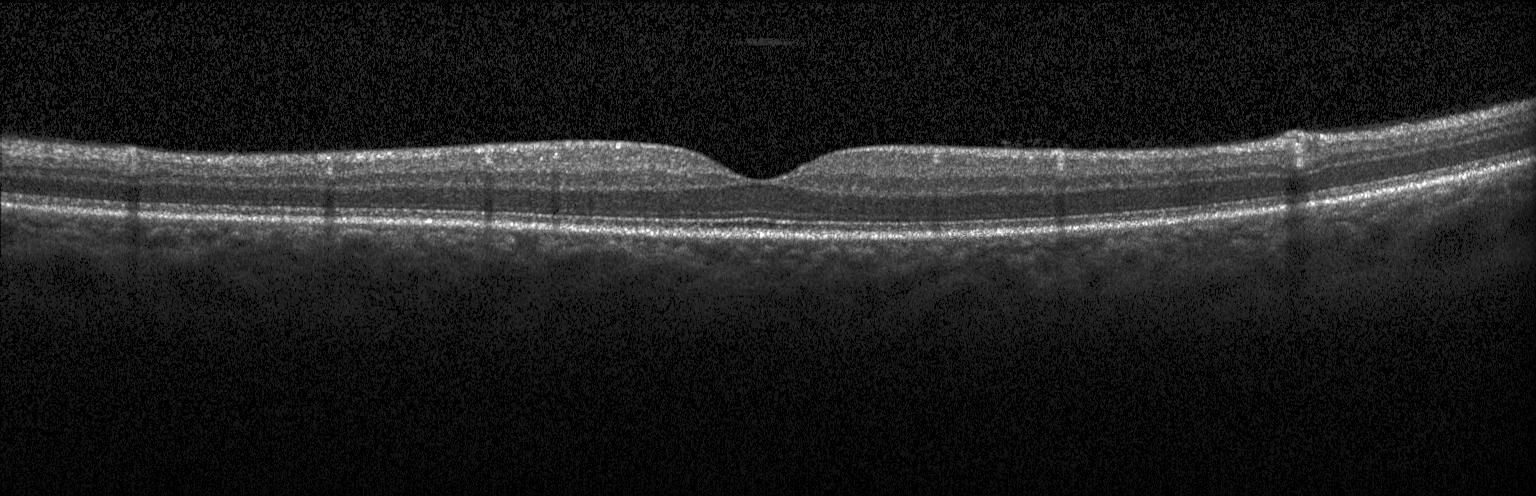 Horizontal scan through the fovea, OCT B-scan, Heidelberg Spectralis — The scan shows no choroidal neovascularization, no diabetic macular edema, and no drusen.